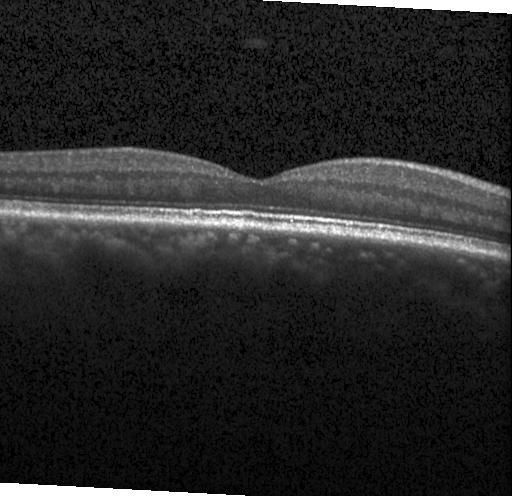

Diagnosis: no CNV, no DME, and no drusen.